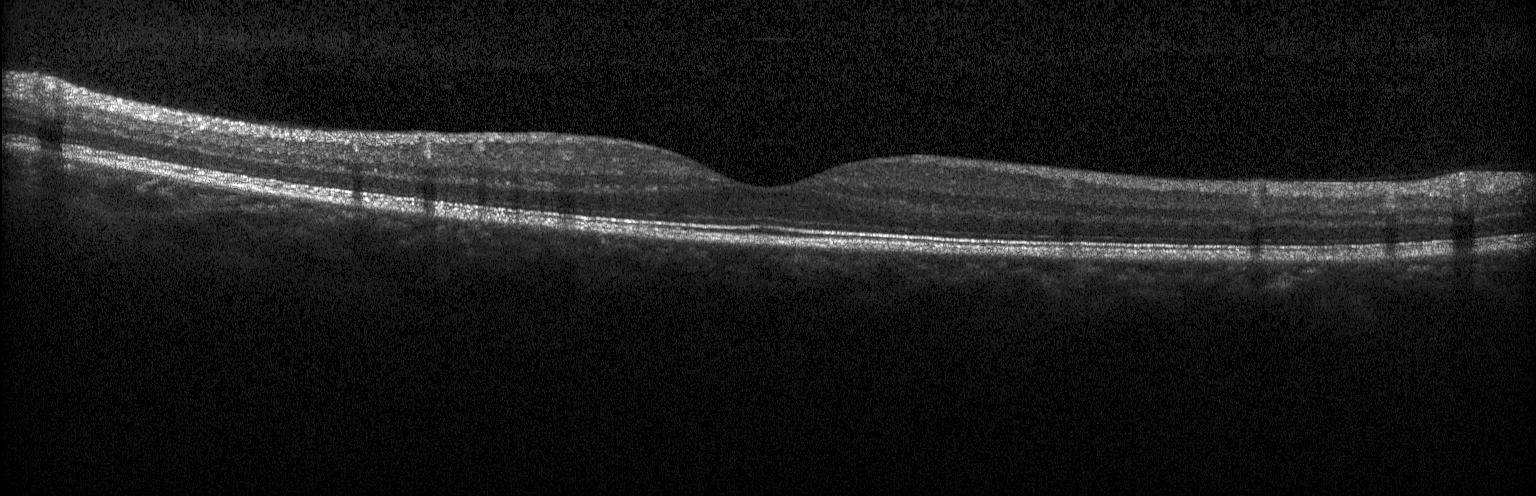 Retinal OCT B-scan. Acquired on a Heidelberg Spectralis. Through the macula. Diagnosis: no choroidal neovascularization, no diabetic macular edema, and no drusen.